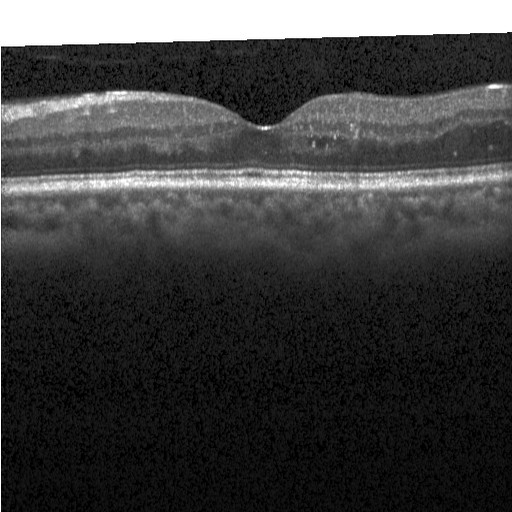 Finding: DME.